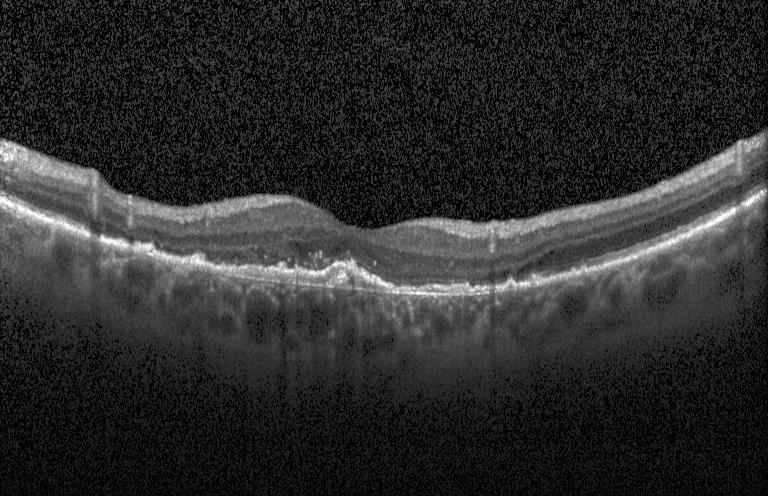 Optical coherence tomography scan — The scan shows choroidal neovascularization (CNV).